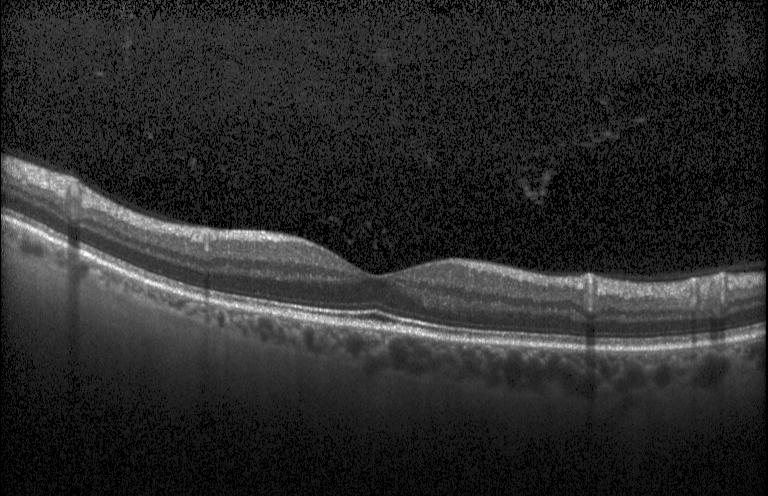

Retinal OCT cross-section. Heidelberg Spectralis OCT system — Impression: neither CNV, DME, nor drusen.